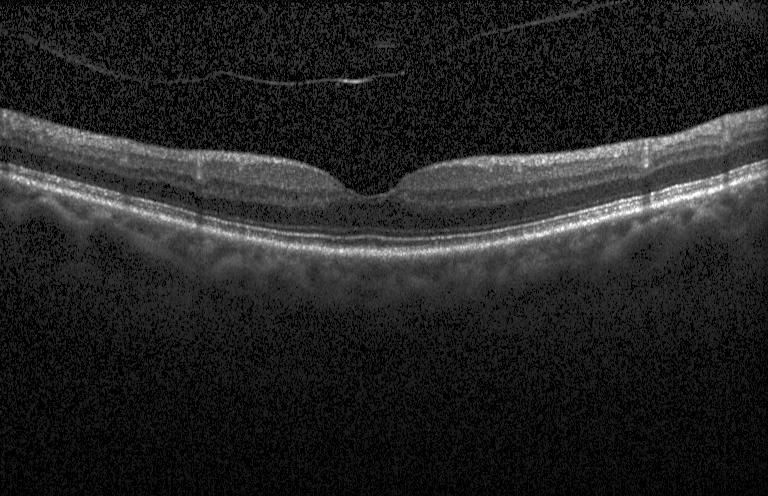
Centered on the fovea; optical coherence tomography B-scan — Finding: no CNV, DME, or drusen.